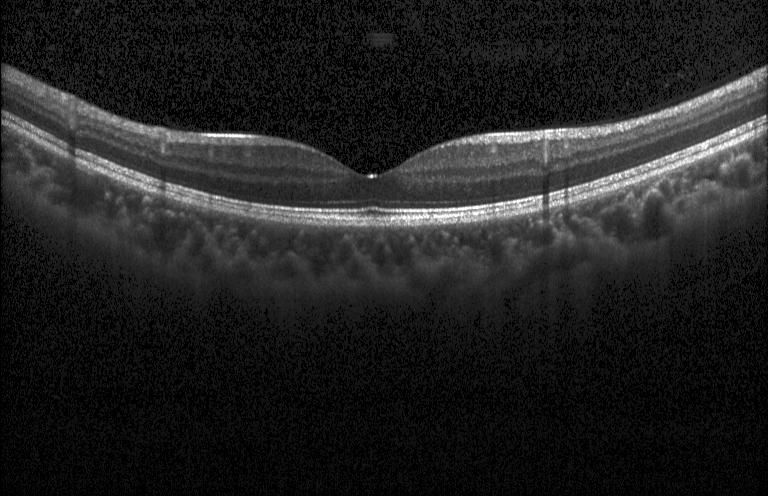
Retinal OCT cross-section.
Impression: no choroidal neovascularization, no diabetic macular edema, and no drusen.